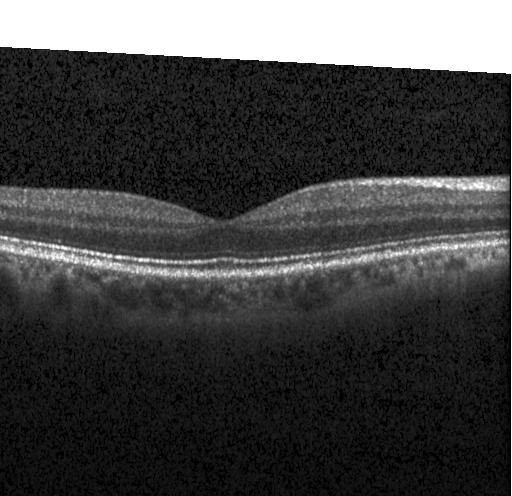 Impression: no evidence of CNV, DME, or drusen.